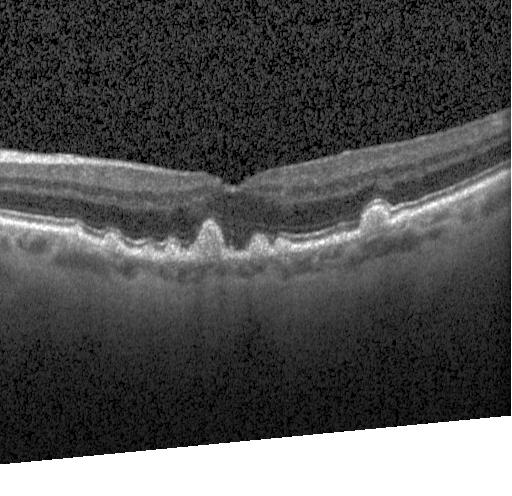

Spectral-domain optical coherence tomography, OCT B-scan, instrument: Heidelberg Spectralis
Diagnosis: multiple drusen.